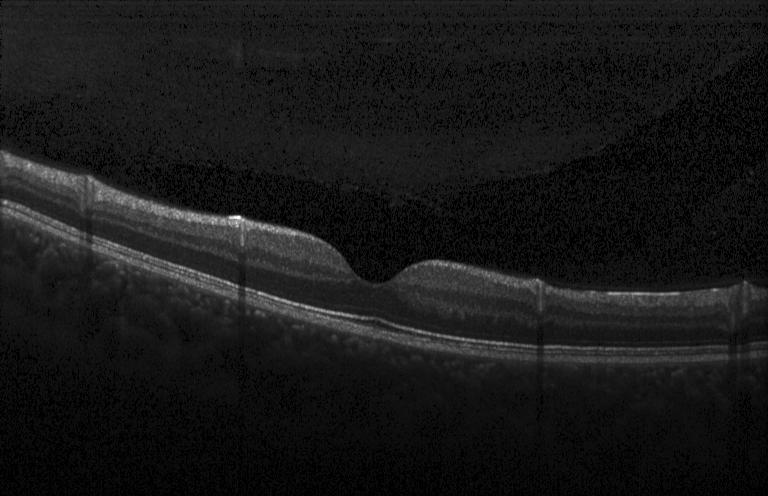

SD-OCT · through the macula · OCT line scan — OCT finding: no choroidal neovascularization, no diabetic macular edema, and no drusen.